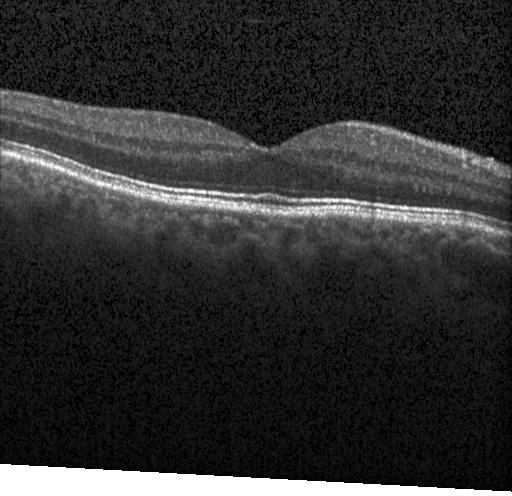
Retinal OCT cross-section showing neither CNV, DME, nor drusen.